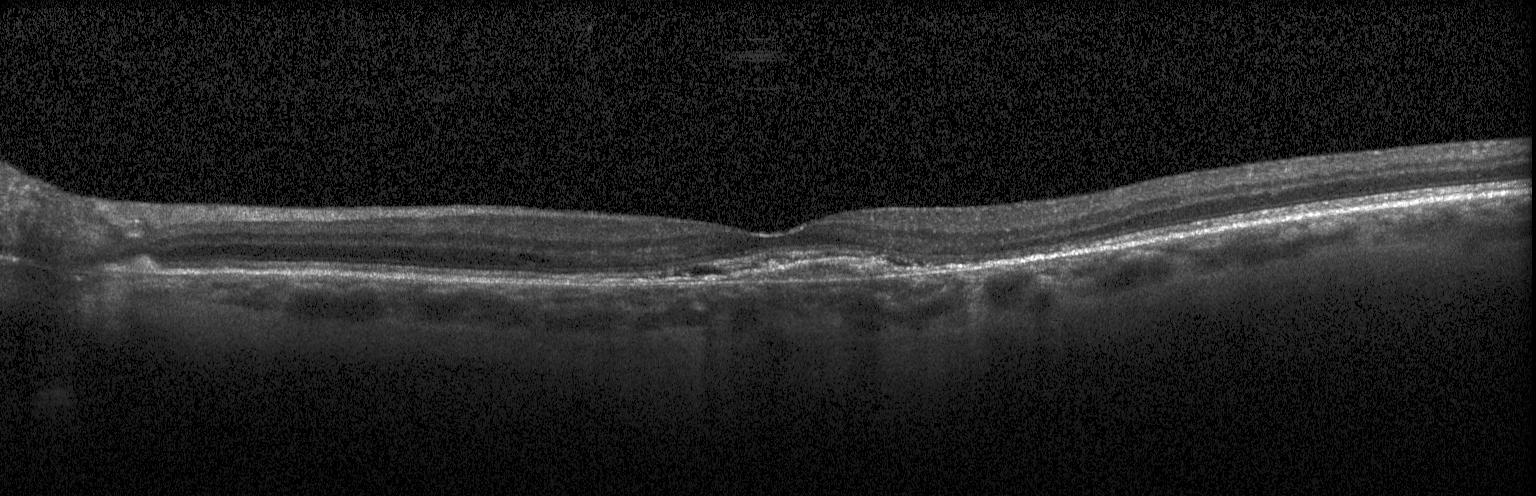
Diagnosis: a choroidal neovascular membrane.